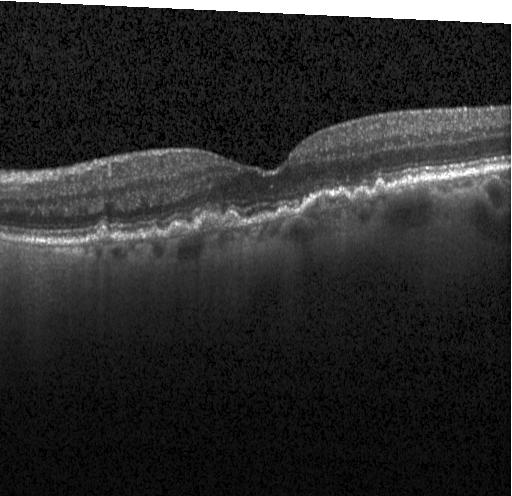
Spectral-domain optical coherence tomography. Horizontal scan through the fovea. OCT line scan. Heidelberg Spectralis OCT system. Impression: drusen.